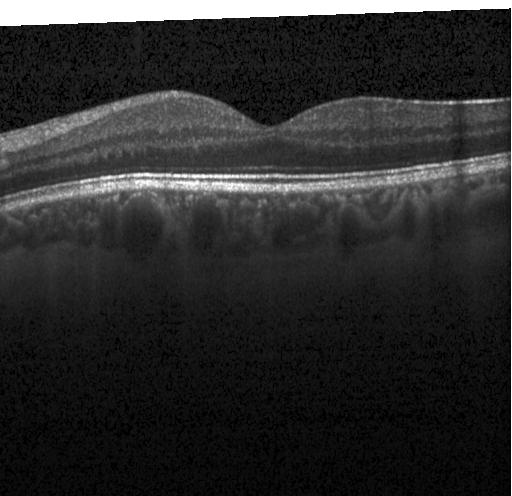
Acquired on a Heidelberg Spectralis. OCT B-scan. Fovea-centered. SD-OCT. Macular OCT: no evidence of choroidal neovascularization, diabetic macular edema, or drusen.